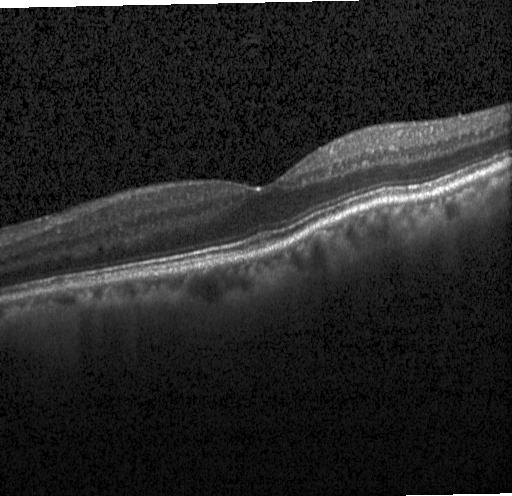 Optical coherence tomography scan. Spectral-domain OCT. Heidelberg Spectralis OCT system. Diagnosis: no evidence of choroidal neovascularization, diabetic macular edema, or drusen.